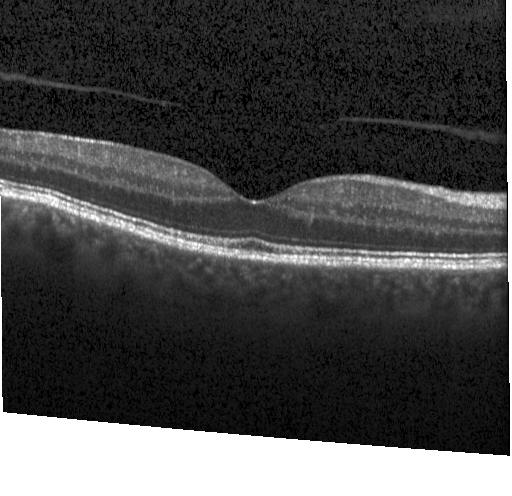 SD-OCT; OCT line scan; acquired on a Heidelberg Spectralis.
This B-scan demonstrates no choroidal neovascularization, diabetic macular edema, or drusen.